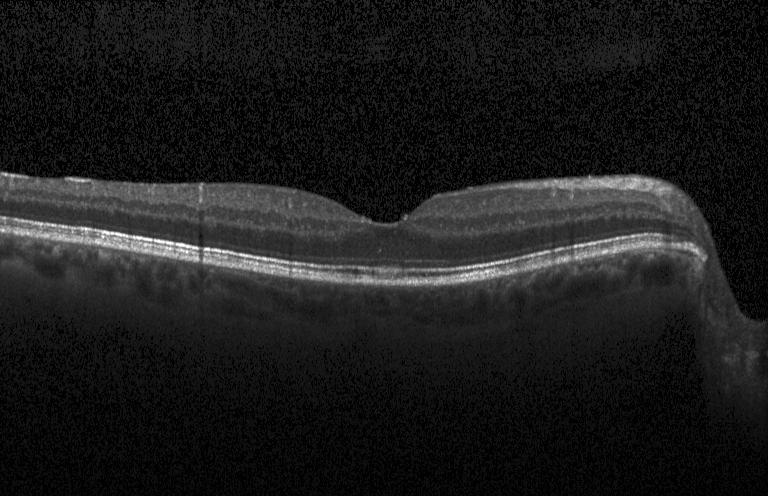

Spectral-domain optical coherence tomography; OCT line scan; fovea-centered. Dx: no evidence of choroidal neovascularization, diabetic macular edema, or drusen.